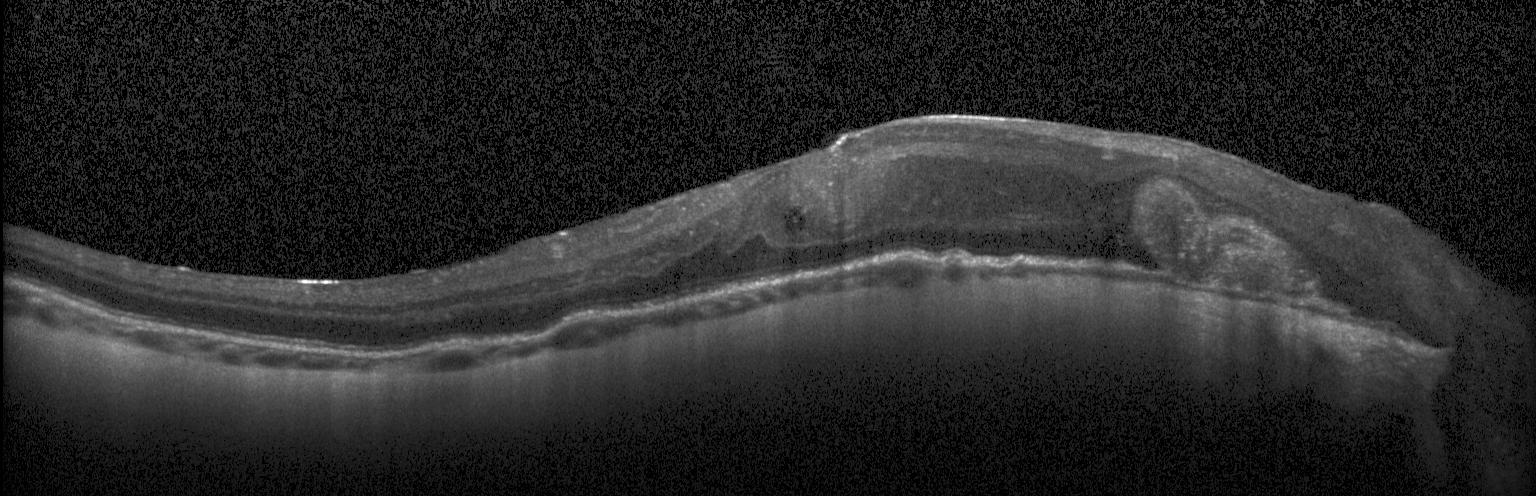

Spectral-domain OCT, optical coherence tomography scan, Heidelberg Spectralis
This B-scan demonstrates diabetic macular edema.